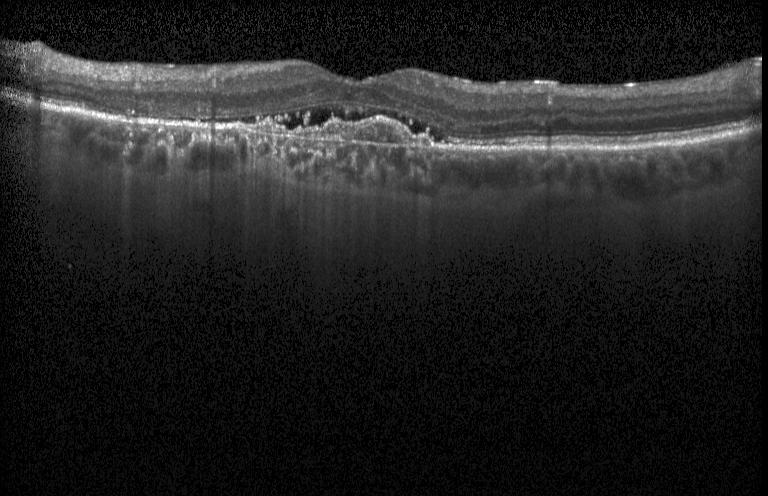

OCT line scan, SD-OCT, instrument: Heidelberg Spectralis — Choroidal neovascularization (CNV).